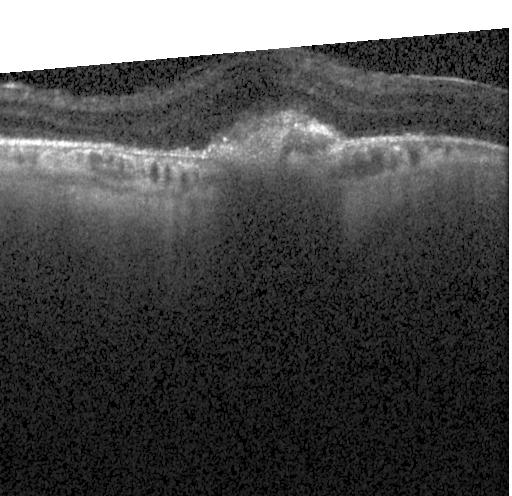 OCT finding: choroidal neovascularization.